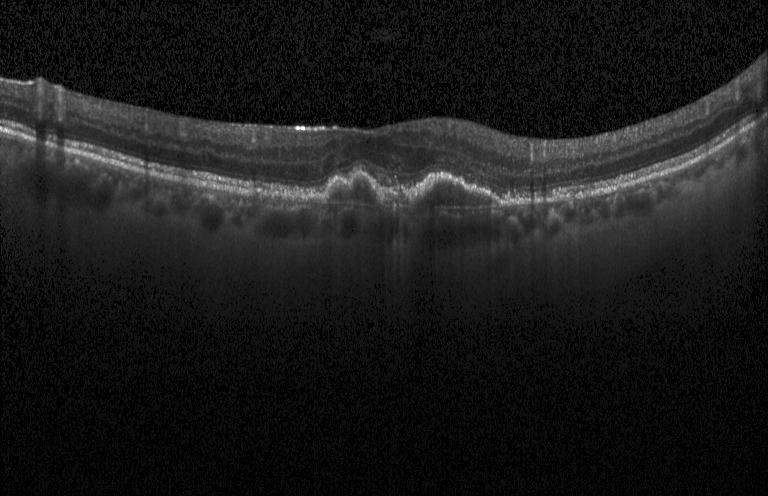 Spectral-domain optical coherence tomography · Heidelberg Spectralis · optical coherence tomography scan · fovea-centered
Finding: a choroidal neovascular membrane.